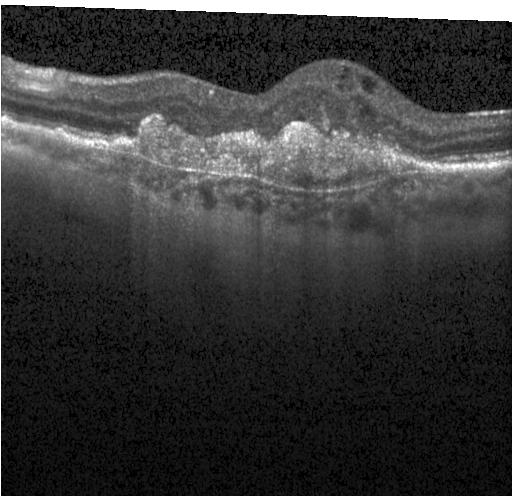

Retinal OCT cross-section — OCT finding: a choroidal neovascular membrane.